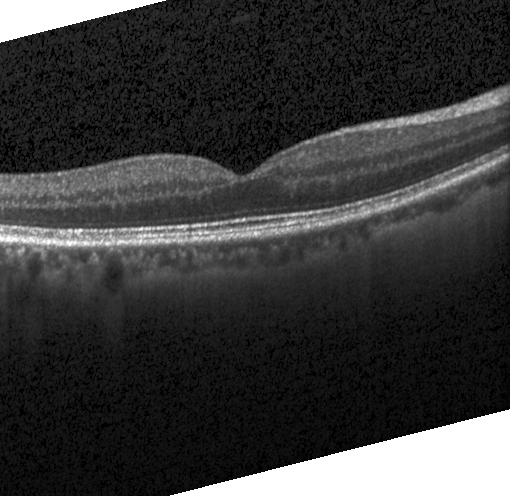 SD-OCT · instrument: Heidelberg Spectralis · centered on the fovea · retinal OCT cross-section.
OCT finding: neither choroidal neovascularization, diabetic macular edema, nor drusen.